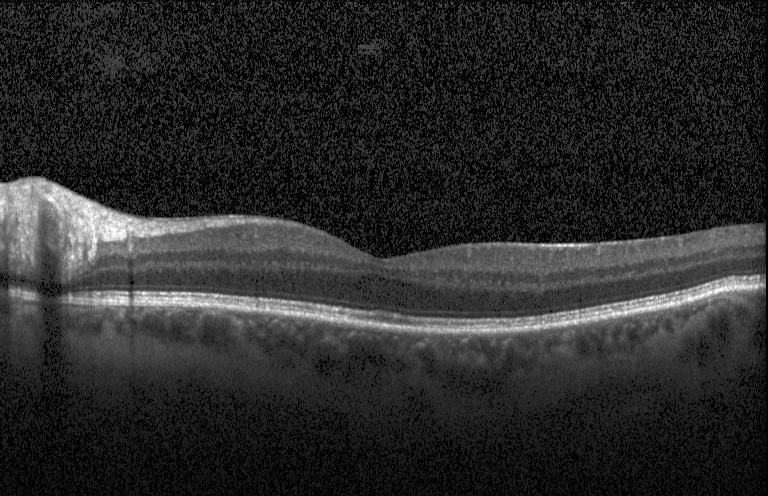
The scan shows no choroidal neovascularization, no diabetic macular edema, and no drusen.